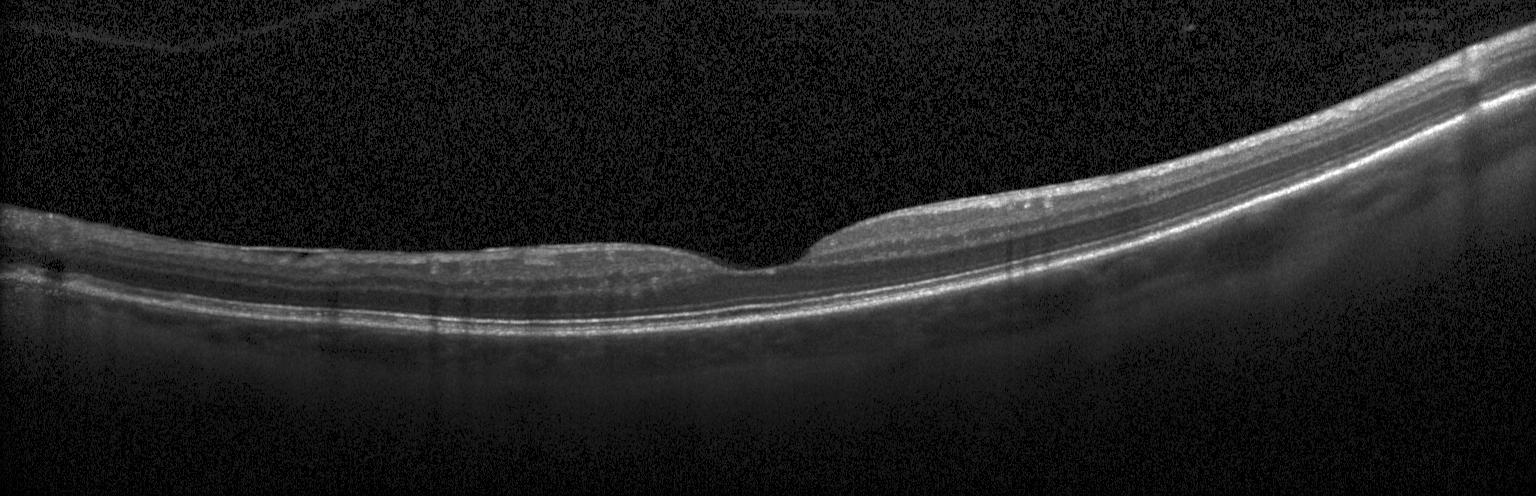

Heidelberg Spectralis OCT system; macular scan; spectral-domain optical coherence tomography; retinal OCT B-scan
Diagnosis: neither CNV, DME, nor drusen.